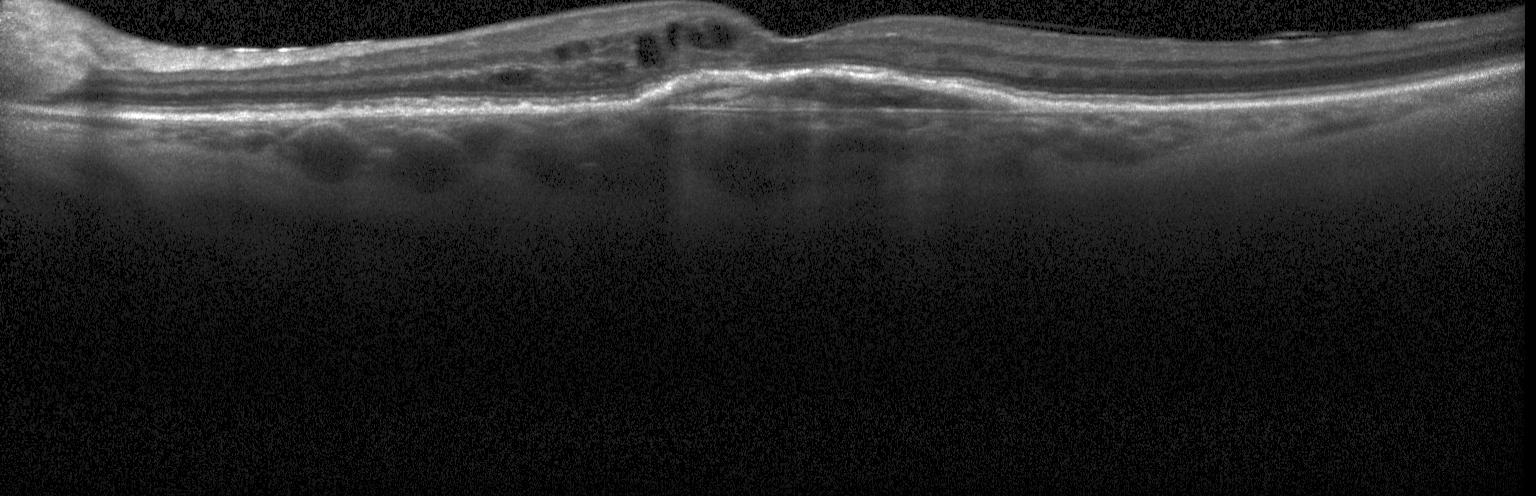 Horizontal scan through the fovea. Retinal OCT cross-section. Instrument: Heidelberg Spectralis. Finding: a choroidal neovascular membrane.